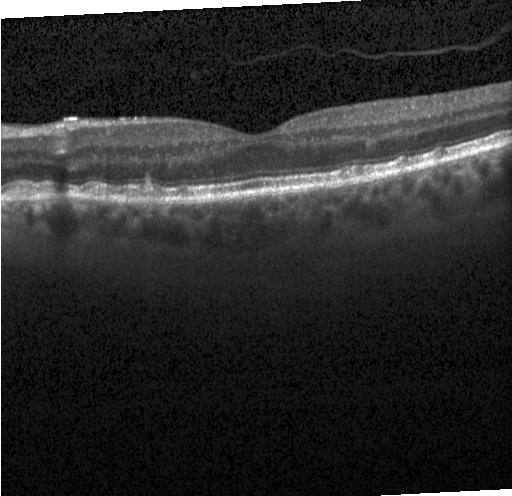 The scan shows sub-RPE drusenoid deposits.